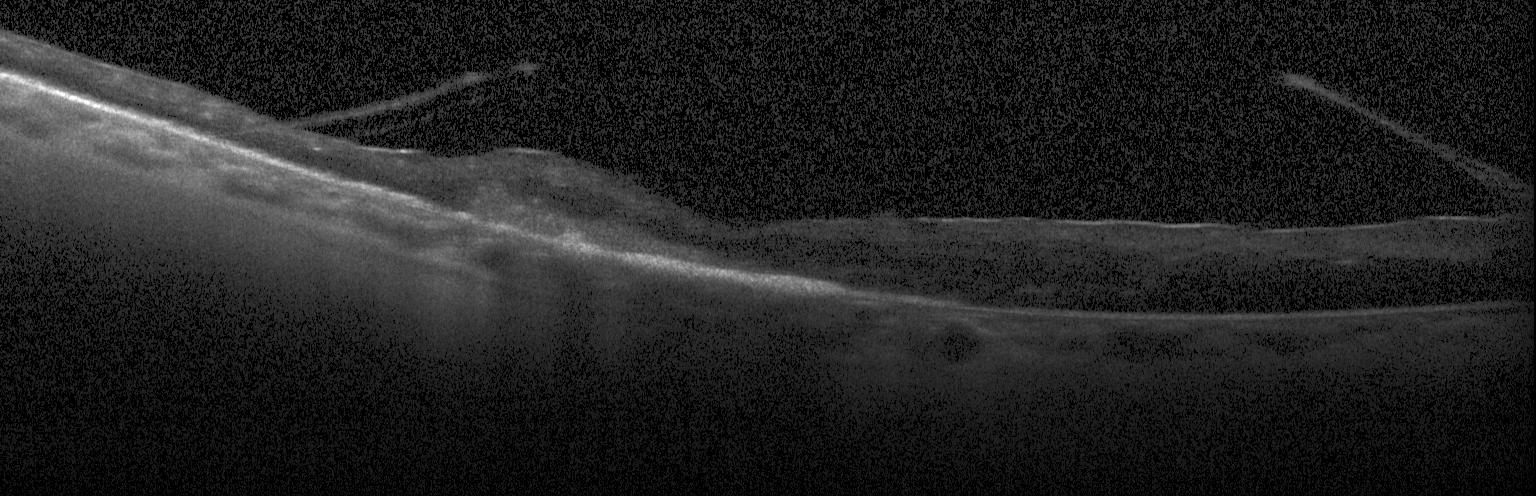 Horizontal scan through the fovea · spectral-domain optical coherence tomography · Heidelberg Spectralis OCT system · optical coherence tomography scan. Choroidal neovascularization (CNV).